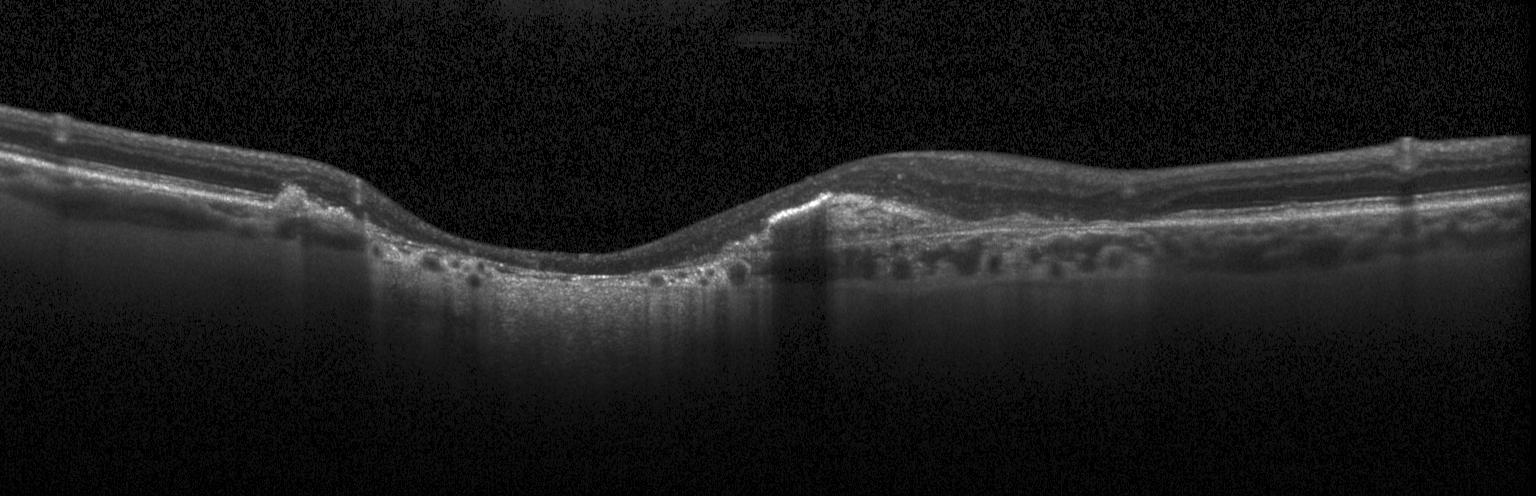

Instrument: Heidelberg Spectralis. Spectral-domain optical coherence tomography. Optical coherence tomography scan. Centered on the fovea. Diagnosis: CNV.